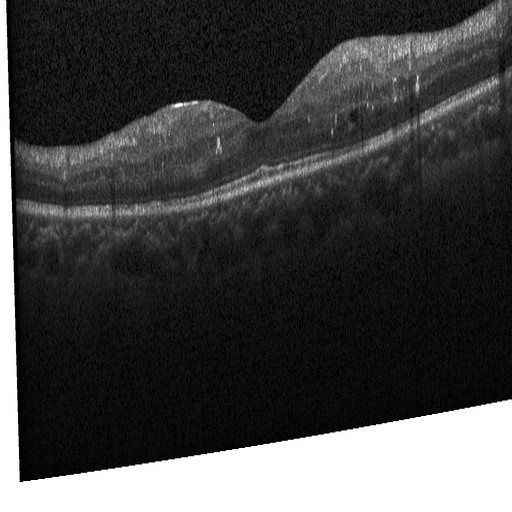

Optical coherence tomography B-scan, spectral-domain optical coherence tomography — OCT finding: diabetic macular edema.